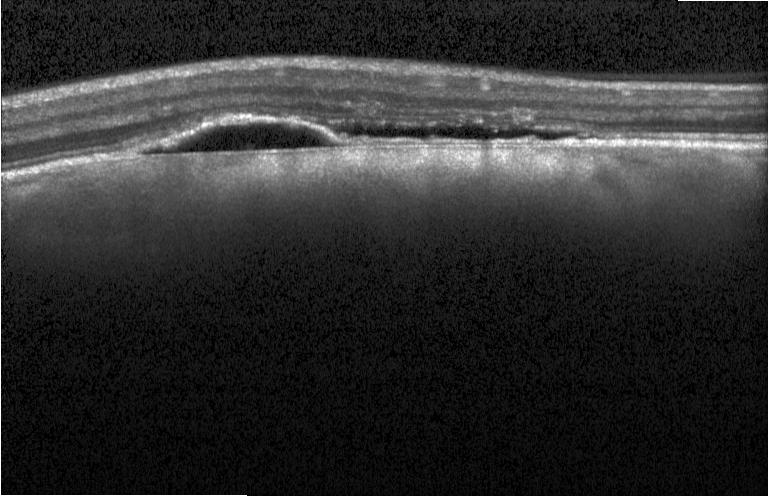

Acquired on a Heidelberg Spectralis, optical coherence tomography B-scan, spectral-domain OCT — Assessment: a choroidal neovascular membrane.